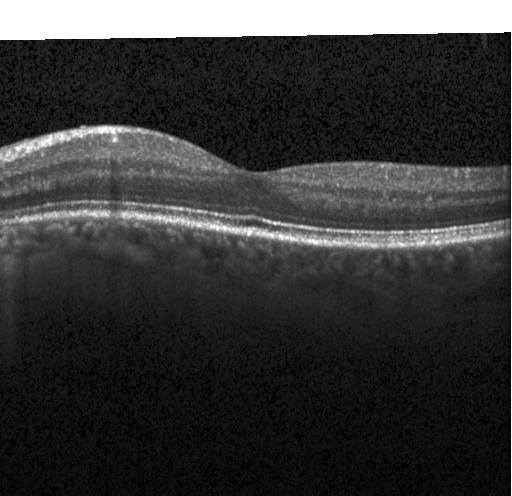
Horizontal scan through the fovea. OCT line scan. Assessment: no evidence of CNV, DME, or drusen.